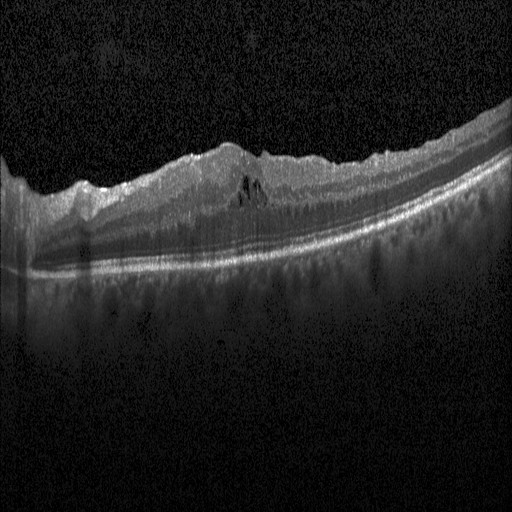
OCT scan showing diabetic macular edema (DME).